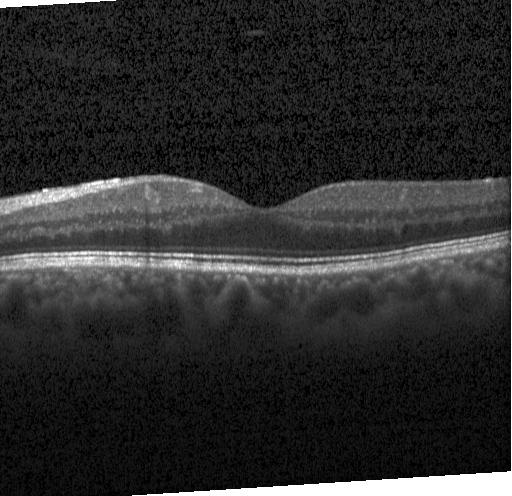

OCT line scan, Heidelberg Spectralis OCT system, through the macula.
Macular OCT: no evidence of CNV, DME, or drusen.